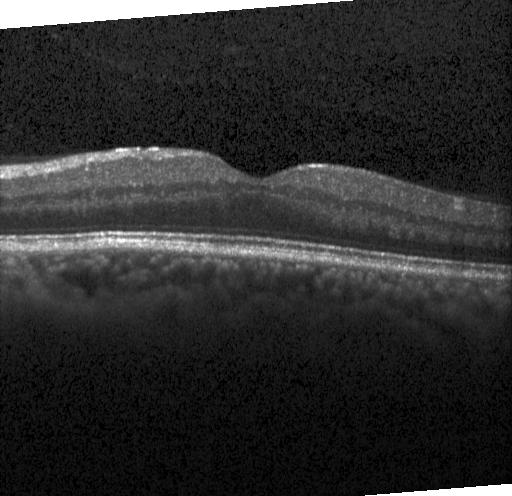
Impression: no CNV, DME, or drusen.